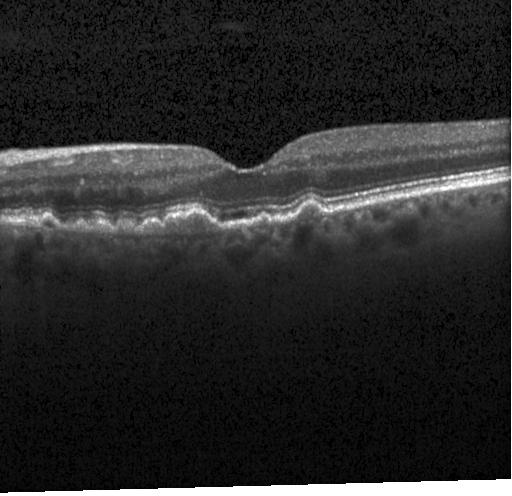
Finding: drusen.